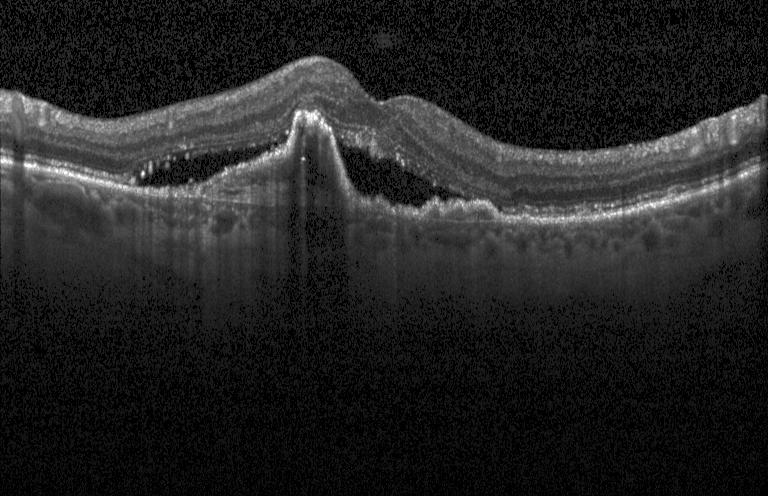

OCT line scan — Dx: CNV.